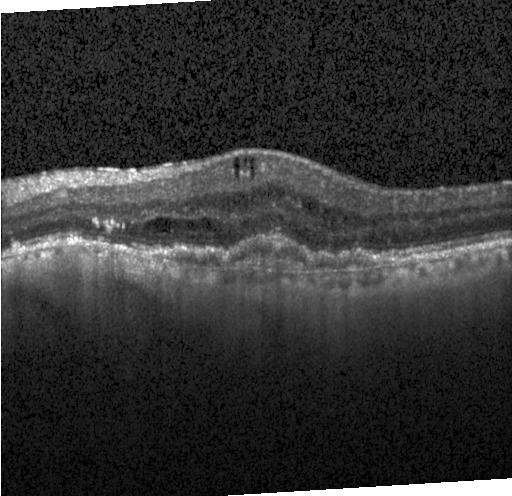

Macular OCT: a choroidal neovascular membrane.